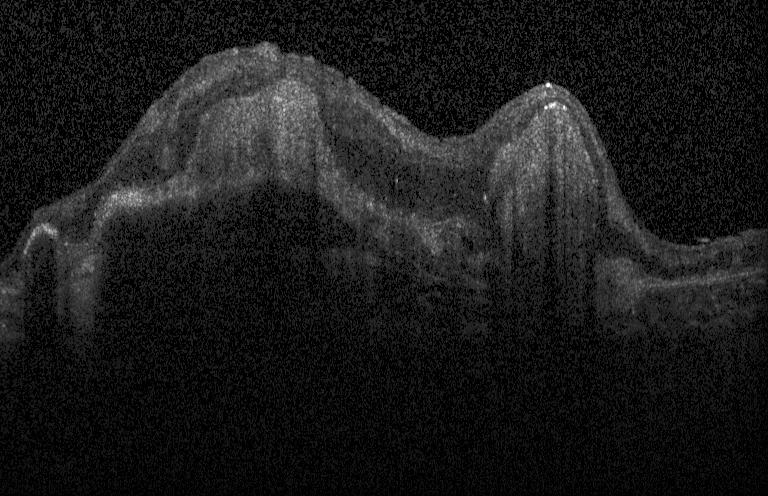
Spectral-domain OCT. Heidelberg Spectralis OCT system. Retinal OCT B-scan.
Diagnosis: a choroidal neovascular membrane.